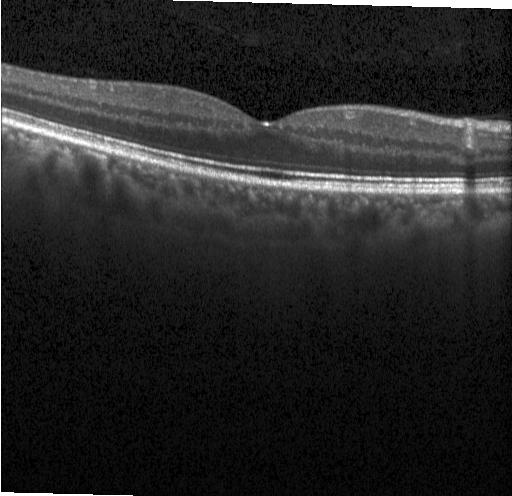
Retinal OCT cross-section · fovea-centered. Assessment: no choroidal neovascularization, diabetic macular edema, or drusen.